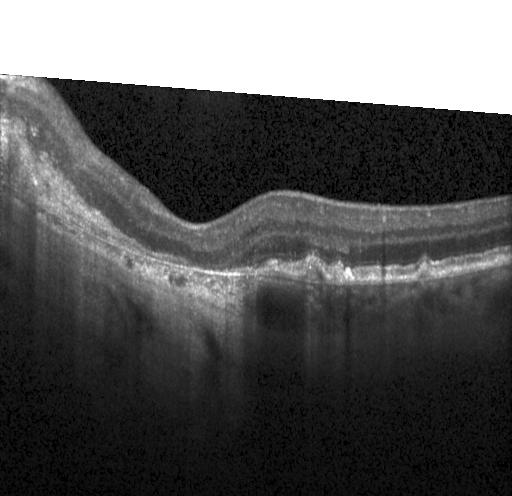 OCT line scan · fovea-centered.
Macular OCT: CNV.